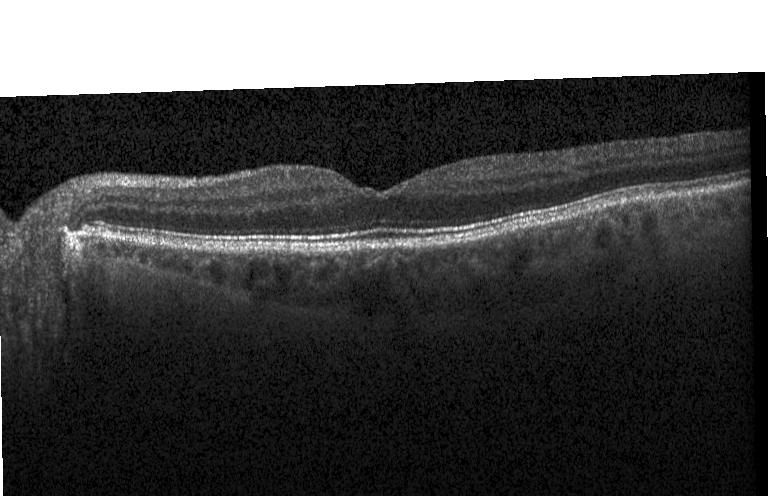 OCT B-scan, acquired on a Heidelberg Spectralis — Finding: neither choroidal neovascularization, diabetic macular edema, nor drusen.